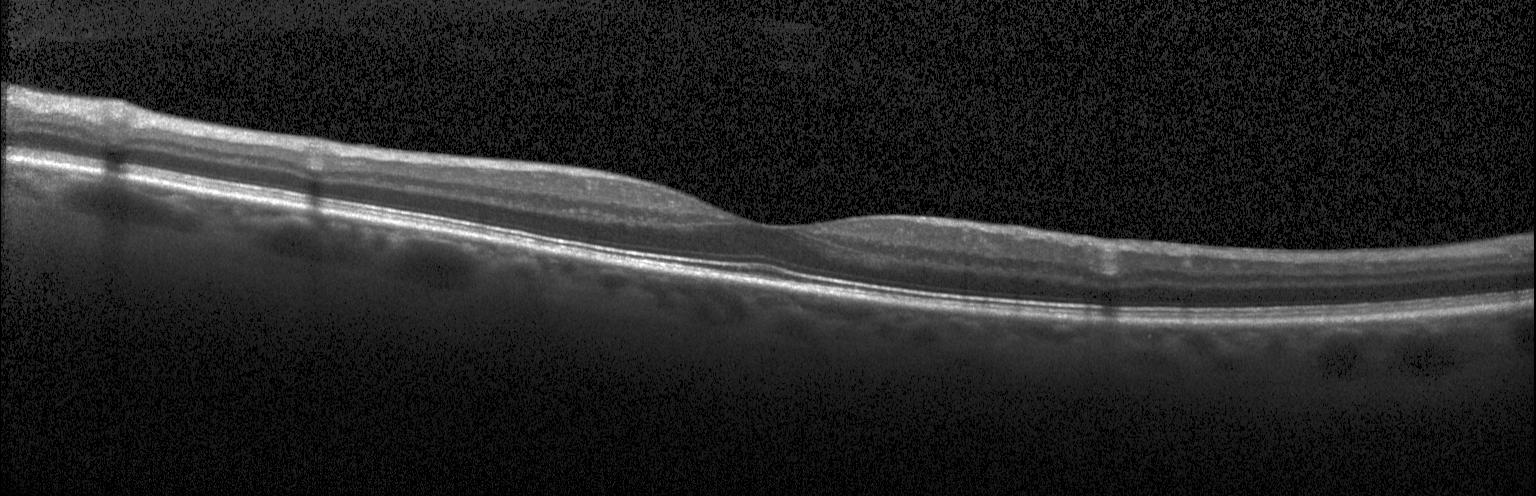 SD-OCT. Heidelberg Spectralis OCT system. OCT B-scan.
Diagnosis: no choroidal neovascularization, diabetic macular edema, or drusen.